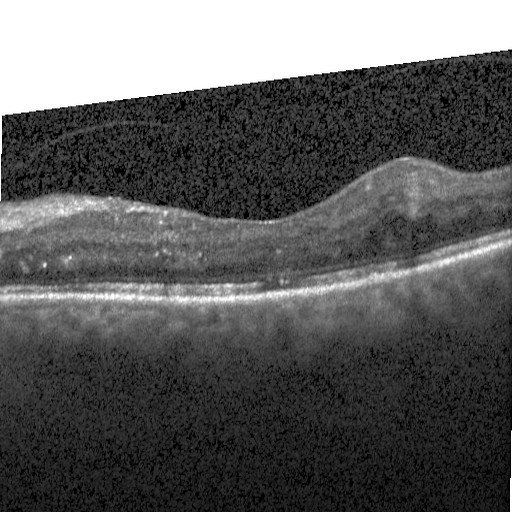 Retinal OCT cross-section showing DME.